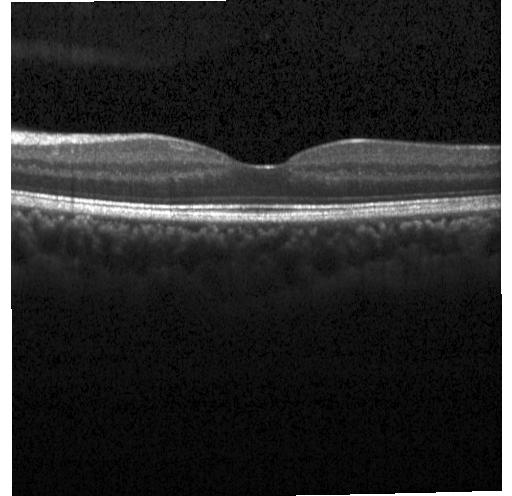 Heidelberg Spectralis OCT system, spectral-domain OCT, retinal OCT cross-section
Impression: no choroidal neovascularization, no diabetic macular edema, and no drusen.